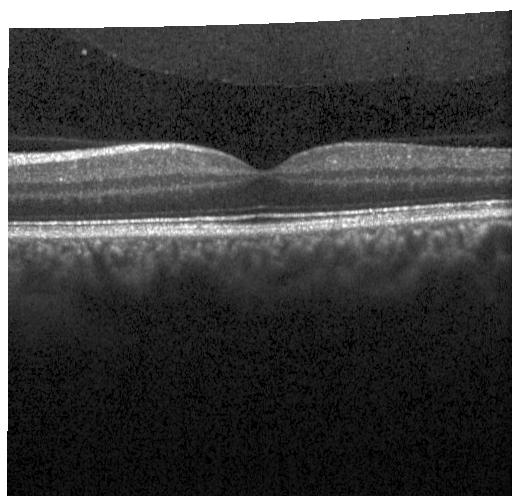
Acquired on a Heidelberg Spectralis, OCT line scan, through the macula — OCT finding: neither CNV, DME, nor drusen.